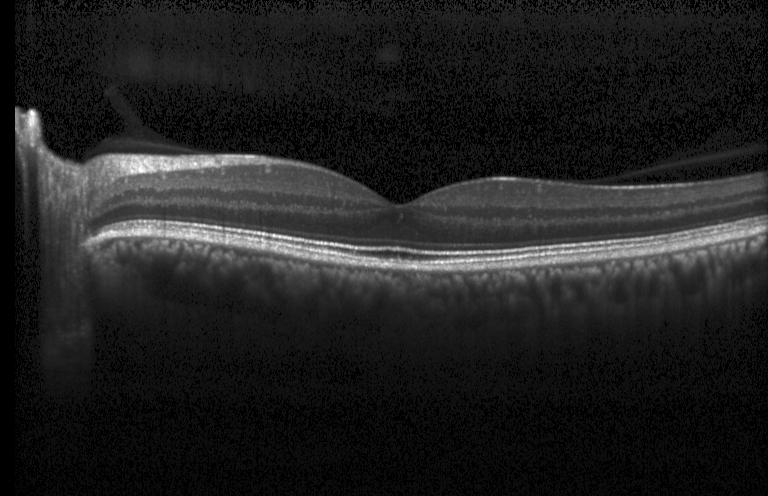 Diagnosis: no evidence of choroidal neovascularization, diabetic macular edema, or drusen.